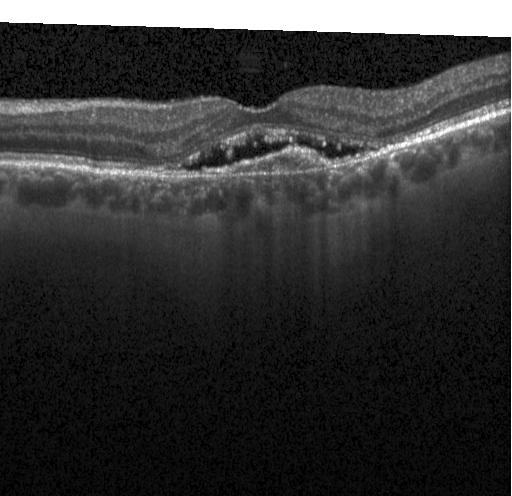
Macular OCT: choroidal neovascularization.